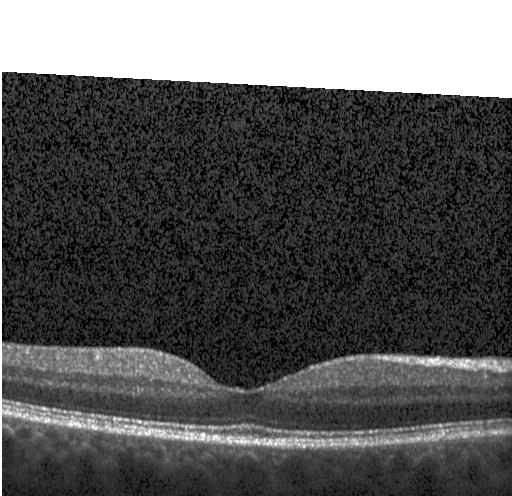
Optical coherence tomography B-scan; fovea-centered. Diagnosis: no CNV, DME, or drusen.